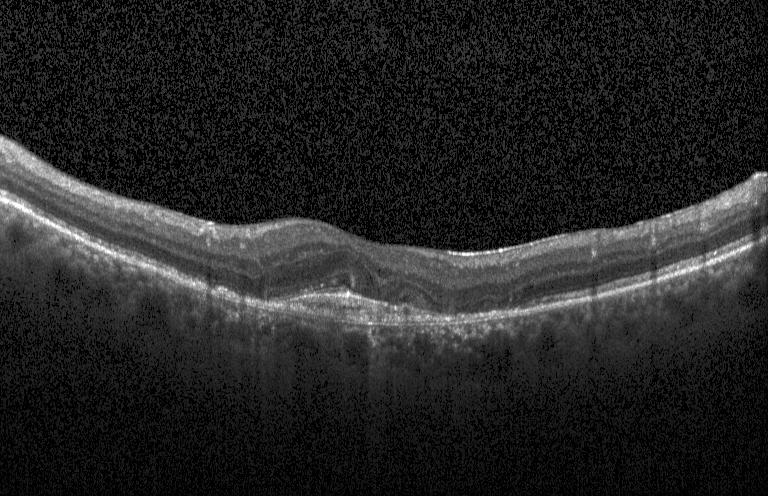
Spectral-domain OCT B-scan: a choroidal neovascular membrane.